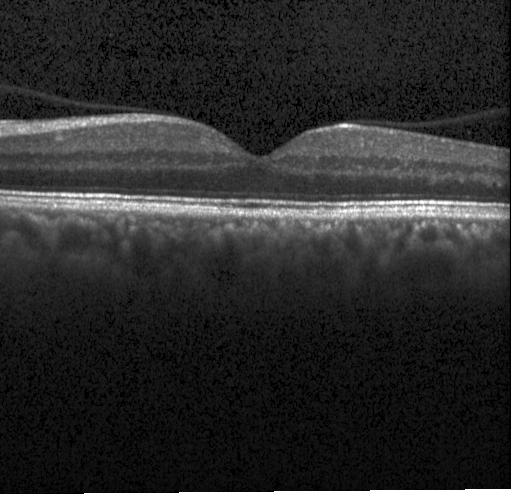 Through the macula · optical coherence tomography scan · SD-OCT — Finding: no evidence of choroidal neovascularization, diabetic macular edema, or drusen.